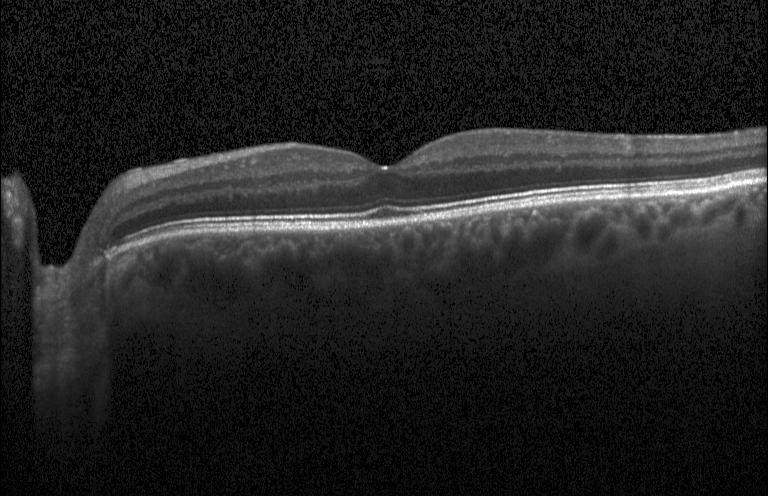
Retinal OCT cross-section, SD-OCT — Impression: no choroidal neovascularization, no diabetic macular edema, and no drusen.